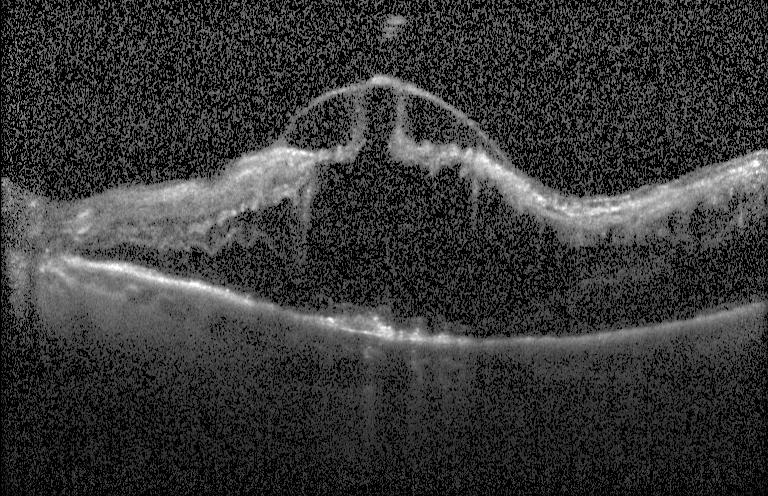 Impression: diabetic macular edema (DME).